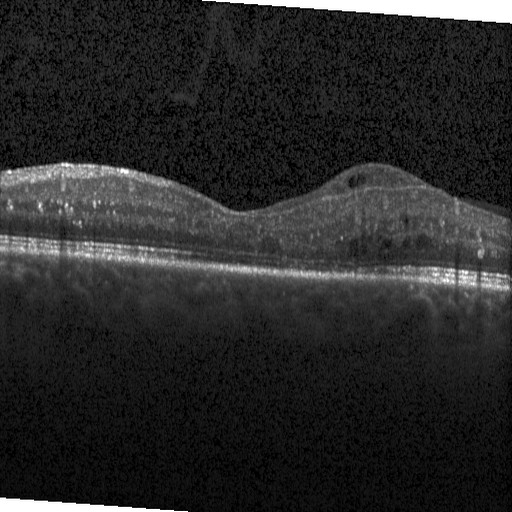

Diabetic macular edema (DME).